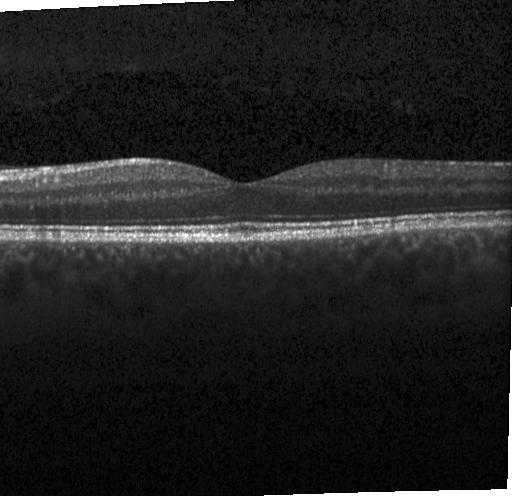
Retinal OCT cross-section. Spectral-domain optical coherence tomography
Impression: no CNV, no DME, and no drusen.